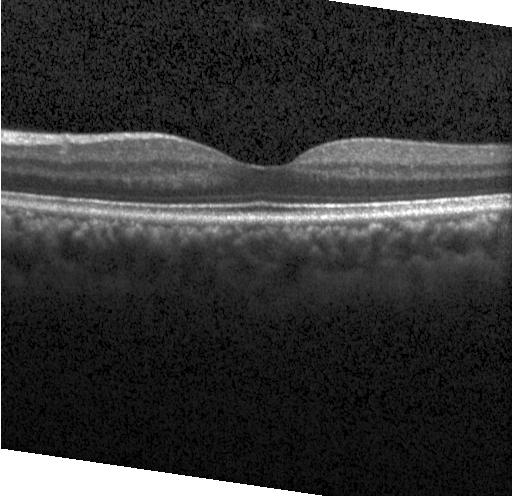
OCT line scan.
Impression: no evidence of choroidal neovascularization, diabetic macular edema, or drusen.